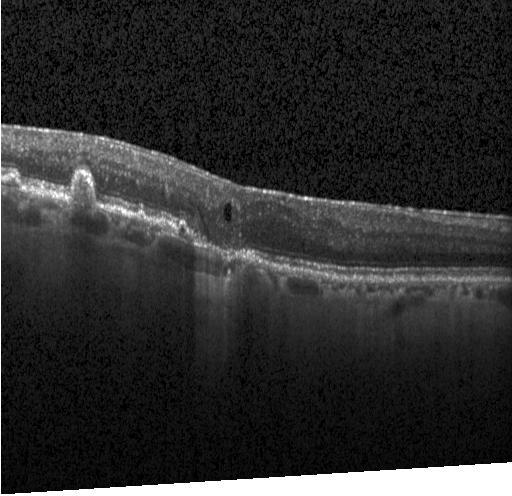 OCT B-scan
Macular OCT: CNV.